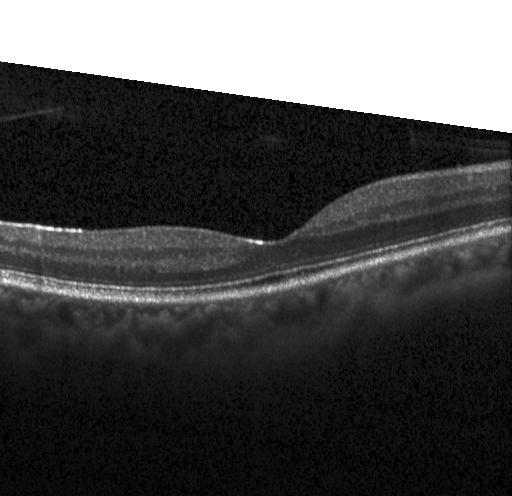
OCT scan showing no choroidal neovascularization, diabetic macular edema, or drusen.